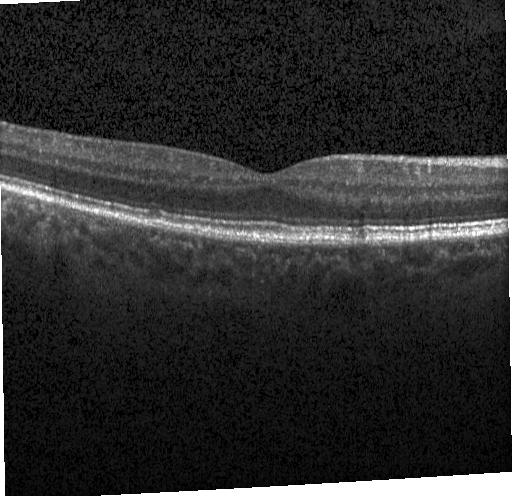
Optical coherence tomography scan. Sub-RPE drusenoid deposits.